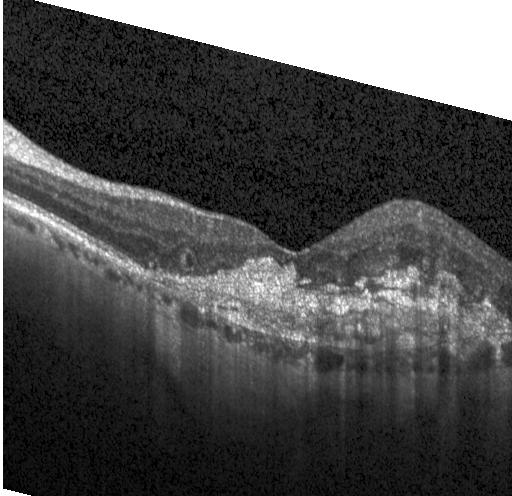 Spectral-domain OCT B-scan: CNV.